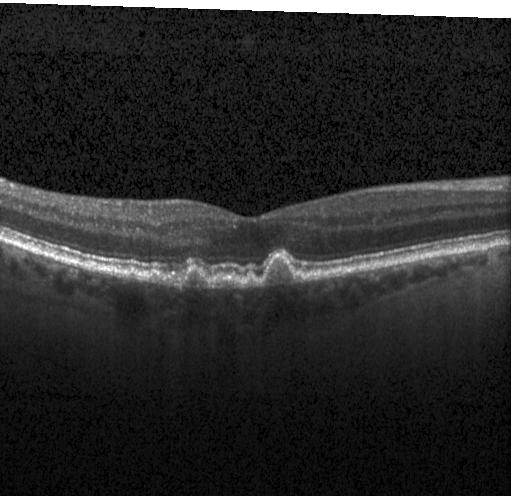

Retinal OCT cross-section
Macular OCT: sub-RPE drusenoid deposits.